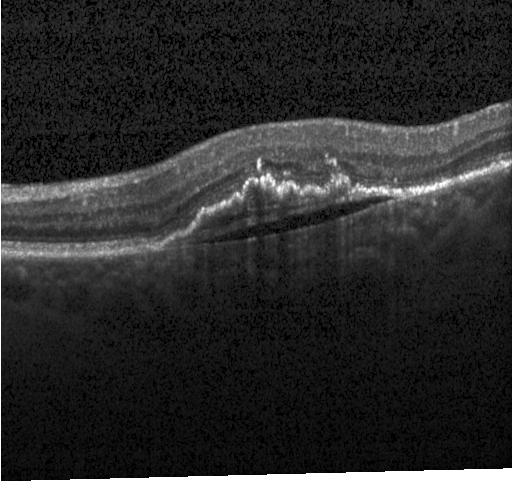

Assessment: a choroidal neovascular membrane.